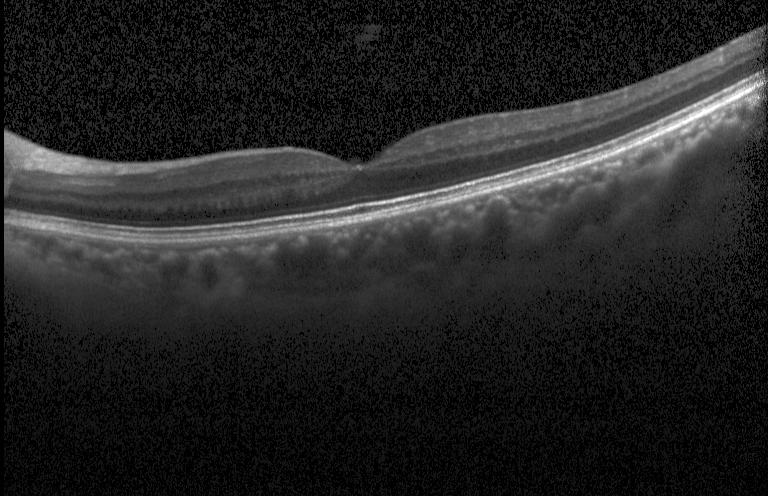
Retinal OCT B-scan; Heidelberg Spectralis OCT system
Finding: no choroidal neovascularization, diabetic macular edema, or drusen.